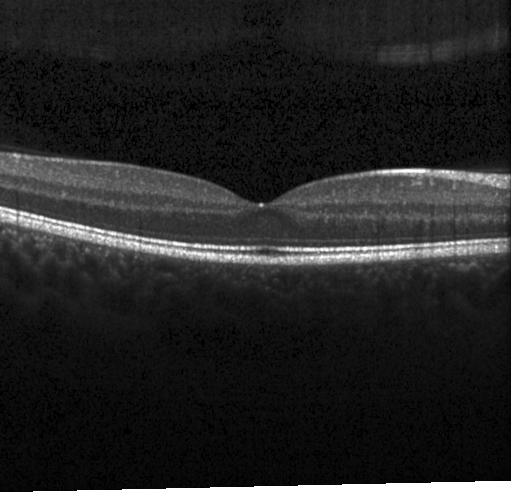

Finding: neither CNV, DME, nor drusen.